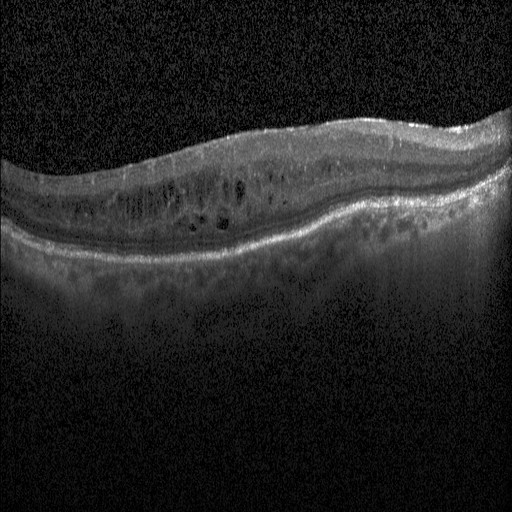 Retinal OCT cross-section showing DME.